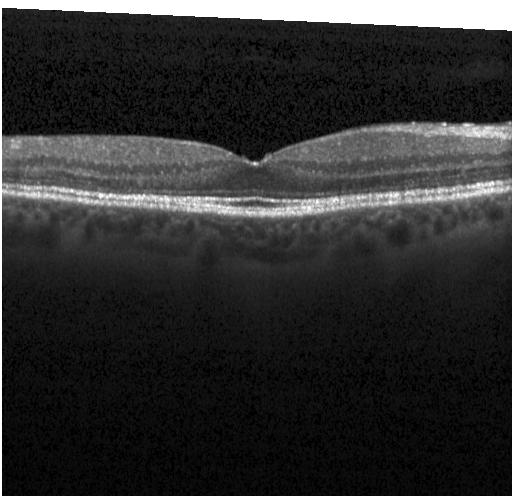

Instrument: Heidelberg Spectralis. Retinal OCT B-scan. OCT finding: no choroidal neovascularization, diabetic macular edema, or drusen.